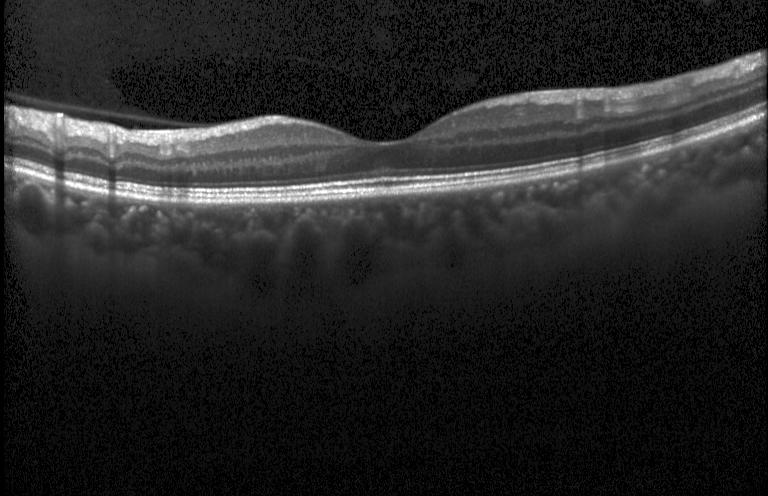

Retinal OCT cross-section · Heidelberg Spectralis OCT system. Diagnosis: no choroidal neovascularization, no diabetic macular edema, and no drusen.